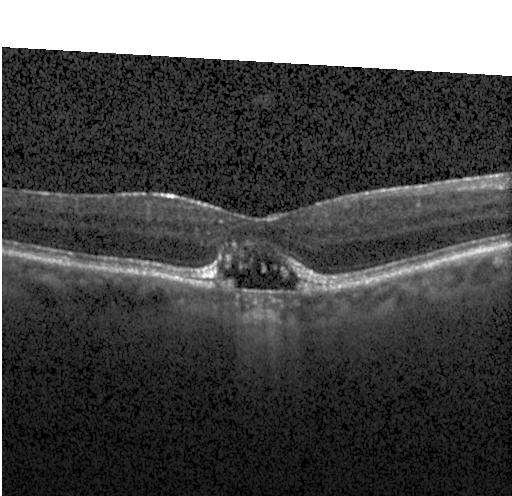

Retinal OCT B-scan · SD-OCT · fovea-centered · acquired on a Heidelberg Spectralis. Impression: a choroidal neovascular membrane.